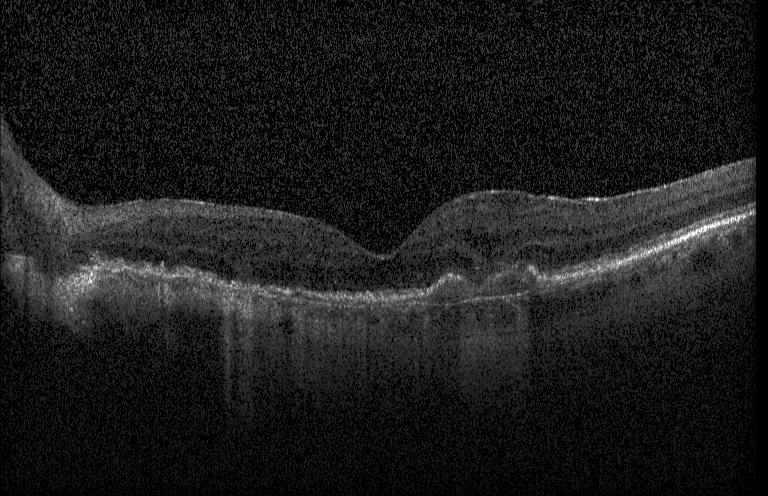

Heidelberg Spectralis. Retinal OCT cross-section — Assessment: choroidal neovascularization.